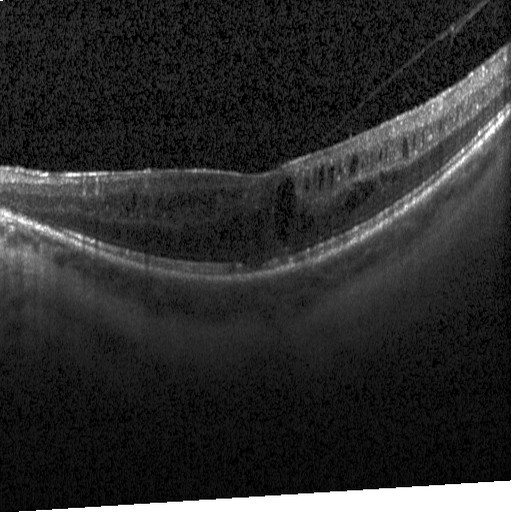
Impression: diabetic macular edema (DME).